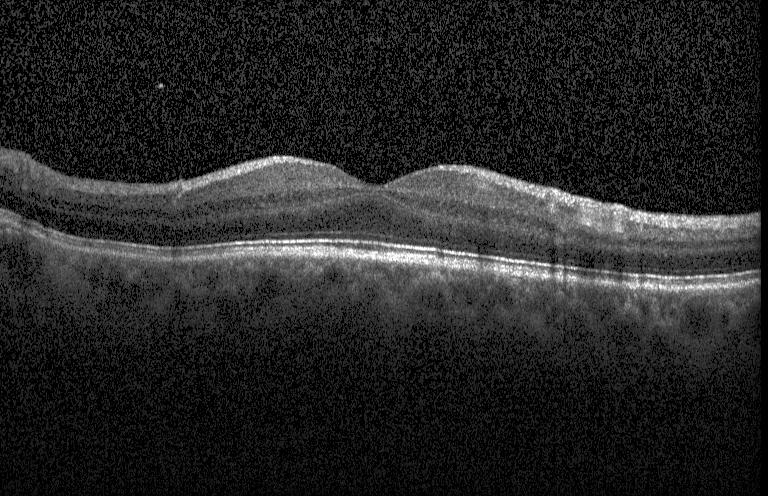 Spectral-domain OCT. Fovea-centered. OCT line scan. Instrument: Heidelberg Spectralis
Finding: no choroidal neovascularization, diabetic macular edema, or drusen.